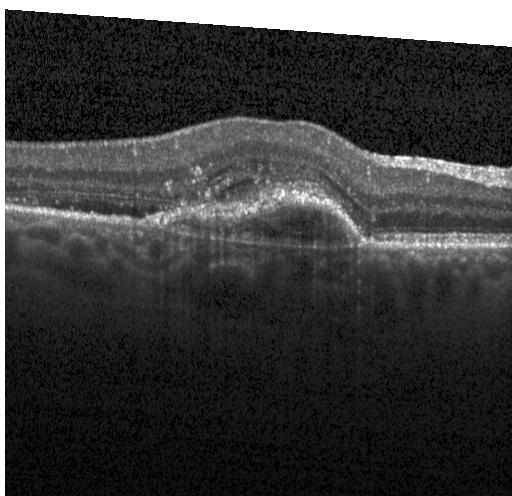

OCT finding: a choroidal neovascular membrane.